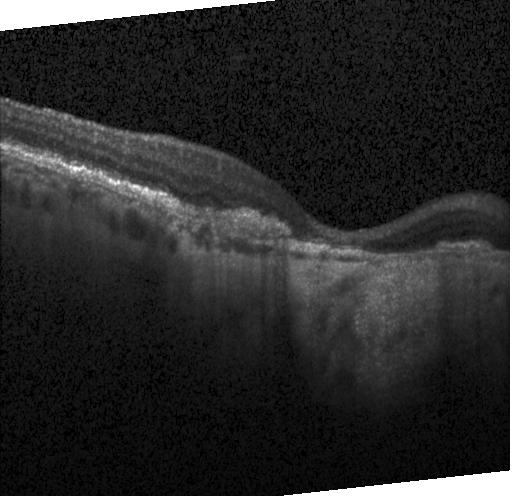 Macular OCT demonstrating choroidal neovascularization.